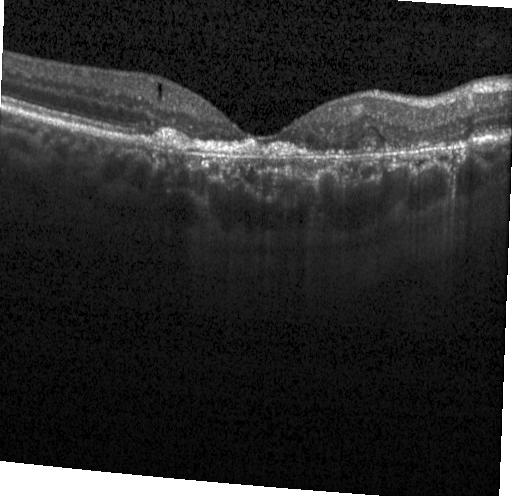

Instrument: Heidelberg Spectralis; SD-OCT; OCT line scan — CNV.